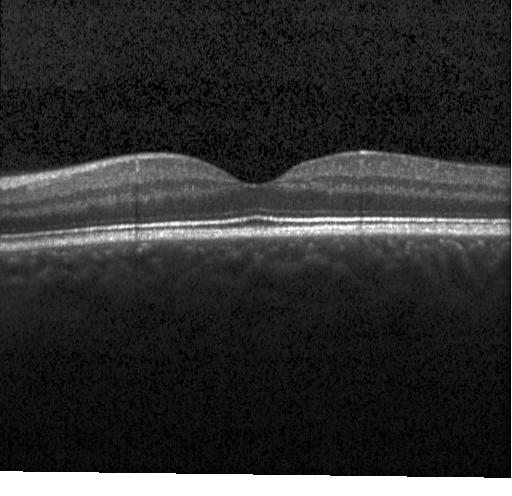
Dx: neither choroidal neovascularization, diabetic macular edema, nor drusen.